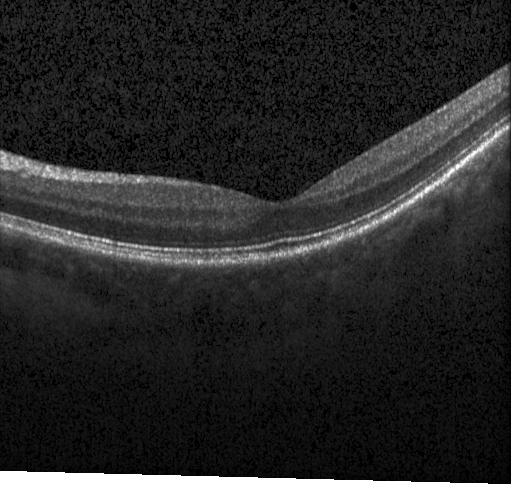

Retinal OCT cross-section; acquired on a Heidelberg Spectralis; macular scan
Diagnosis: no choroidal neovascularization, no diabetic macular edema, and no drusen.